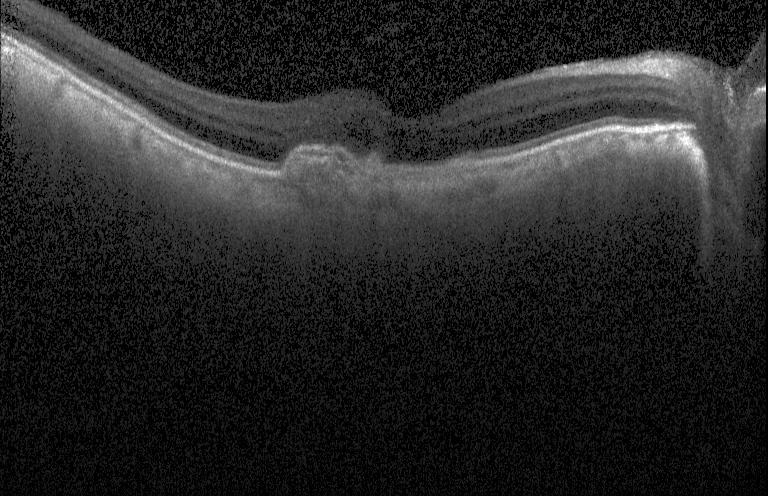

Dx: a choroidal neovascular membrane.